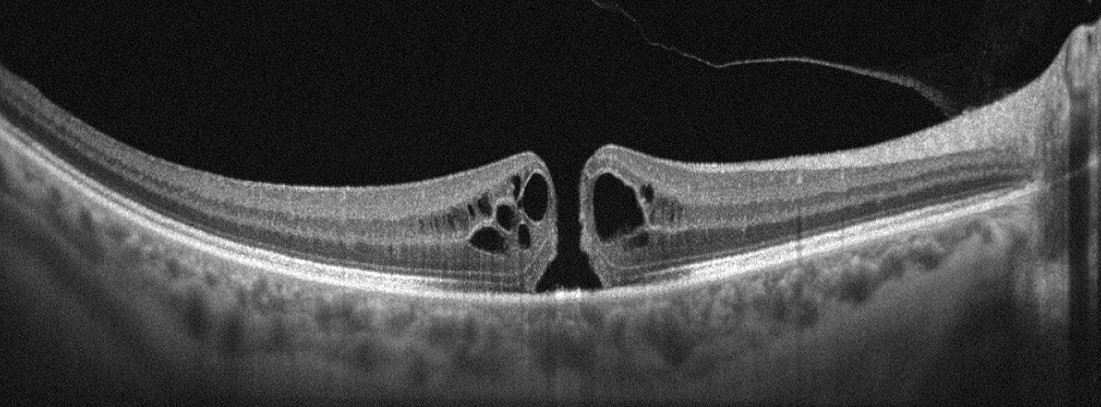

Spectral-domain OCT B-scan: VID.